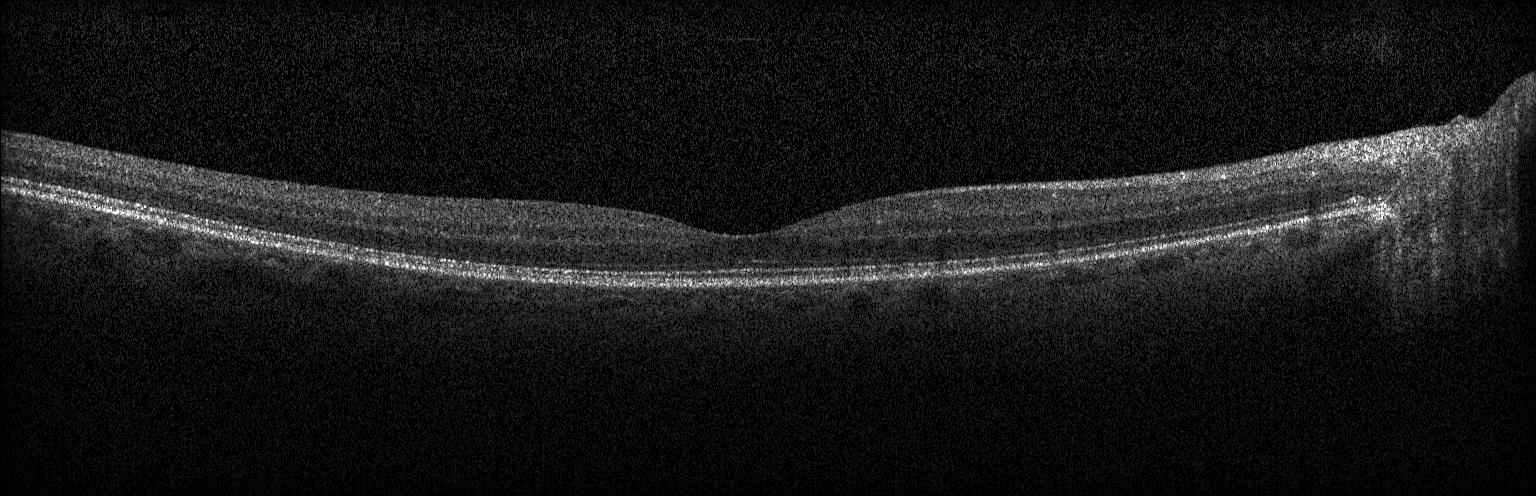

Instrument: Heidelberg Spectralis; OCT B-scan
The scan shows no choroidal neovascularization, diabetic macular edema, or drusen.